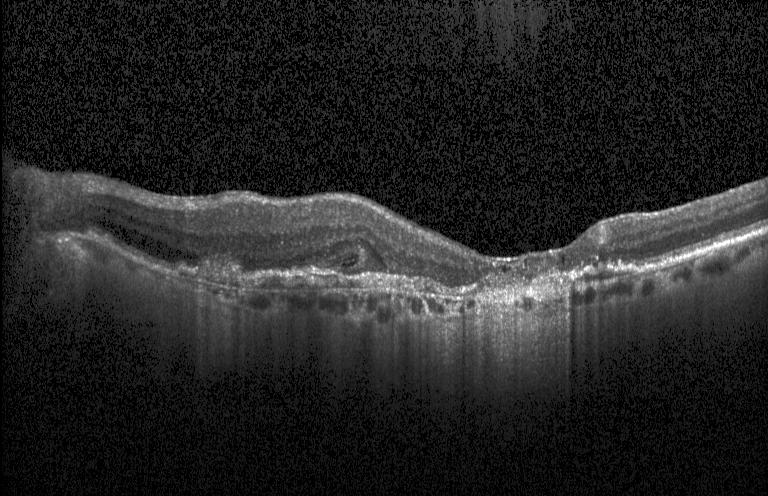 Through the macula, optical coherence tomography scan, spectral-domain OCT
Dx: a choroidal neovascular membrane.